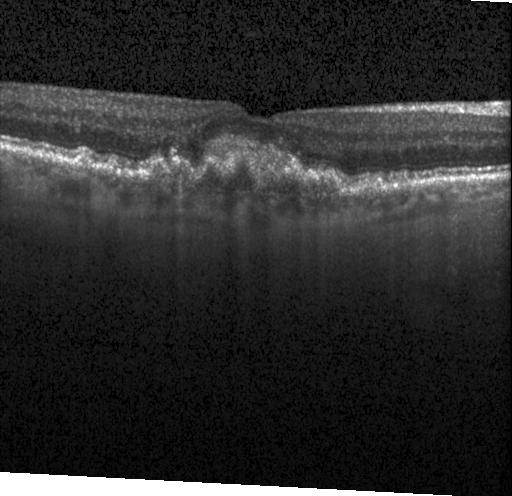
This B-scan demonstrates choroidal neovascularization (CNV).